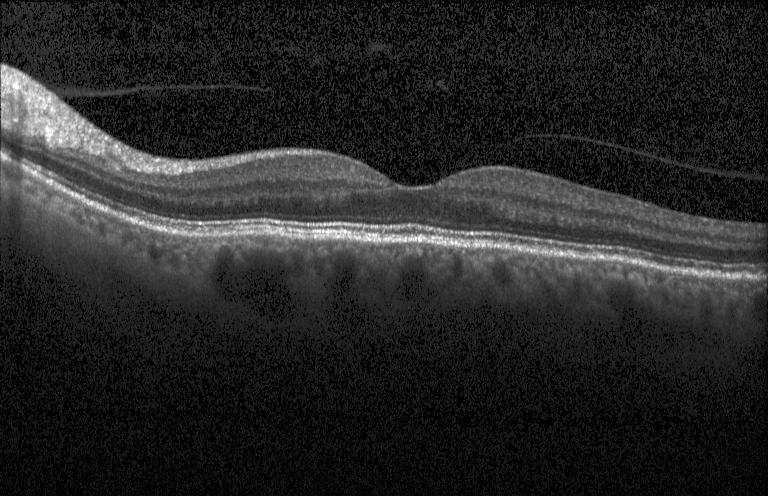 Instrument: Heidelberg Spectralis. Optical coherence tomography scan. Spectral-domain OCT
OCT finding: no CNV, no DME, and no drusen.